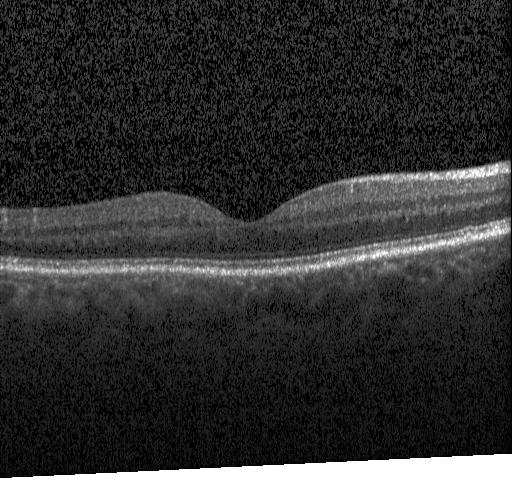
Spectral-domain OCT B-scan: no CNV, no DME, and no drusen.